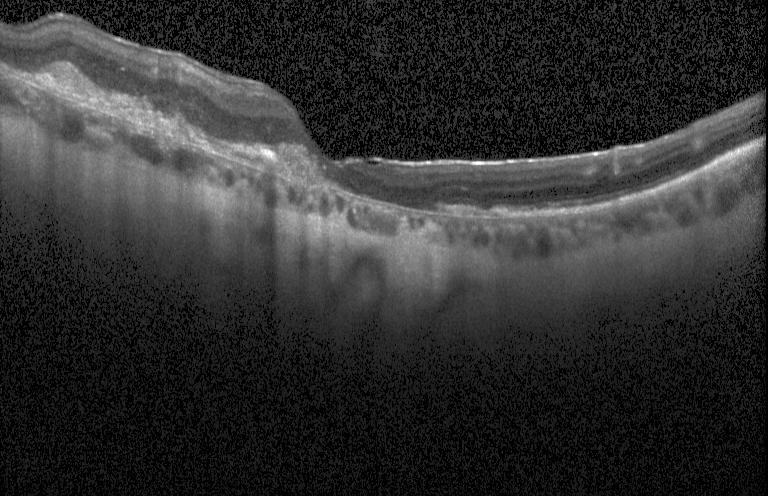
Impression: choroidal neovascularization.